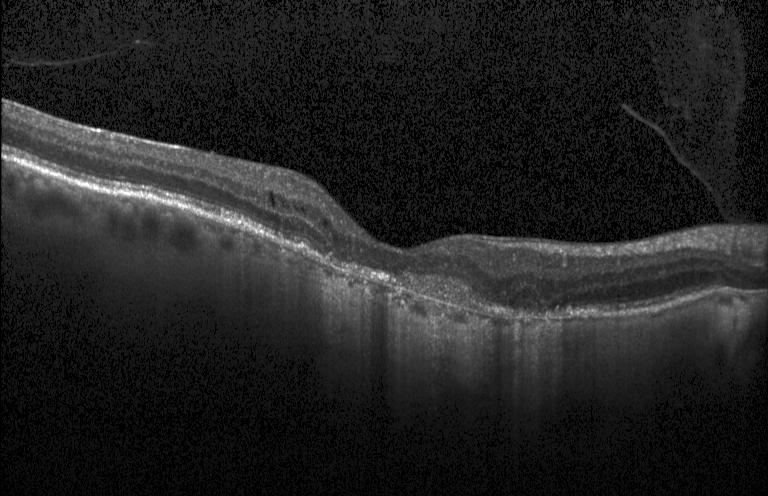

The scan shows choroidal neovascularization.